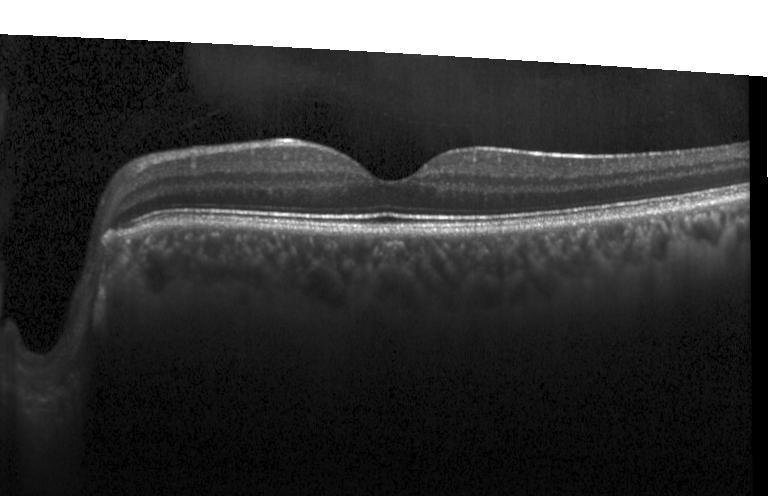
The scan shows no choroidal neovascularization, no diabetic macular edema, and no drusen.